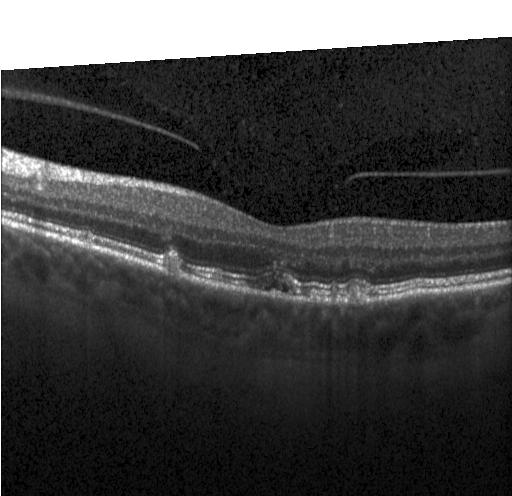

OCT finding: drusen.